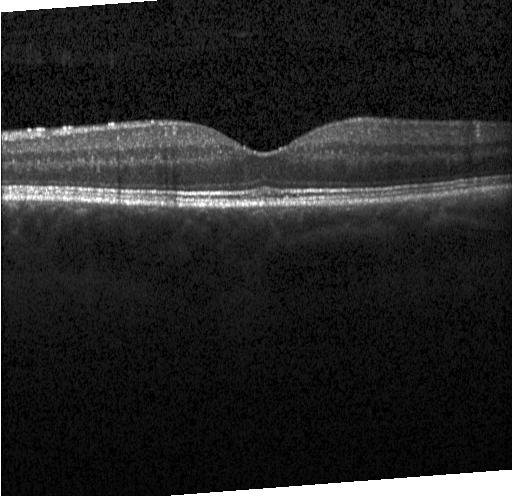 Optical coherence tomography scan
Diagnosis: no choroidal neovascularization, no diabetic macular edema, and no drusen.